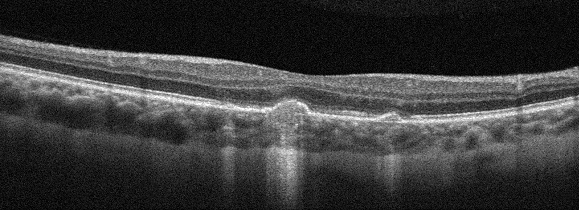
Left eye; OCT B-scan. Diagnosis: age-related macular degeneration.